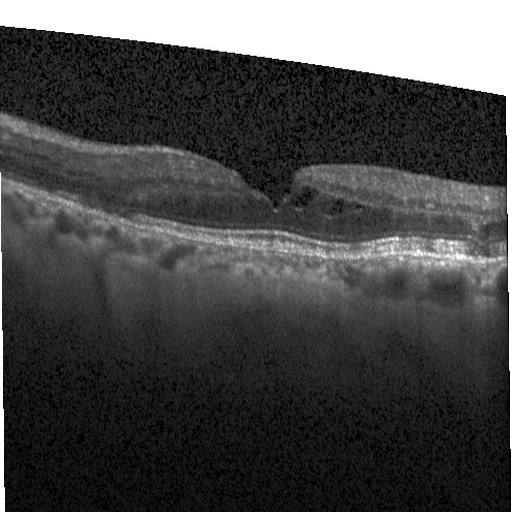
Optical coherence tomography scan, instrument: Heidelberg Spectralis.
Impression: DME.